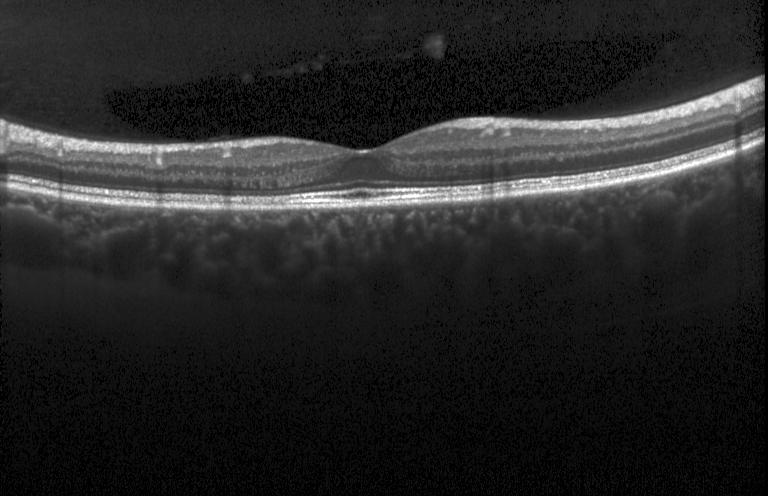

OCT scan showing no choroidal neovascularization, diabetic macular edema, or drusen.